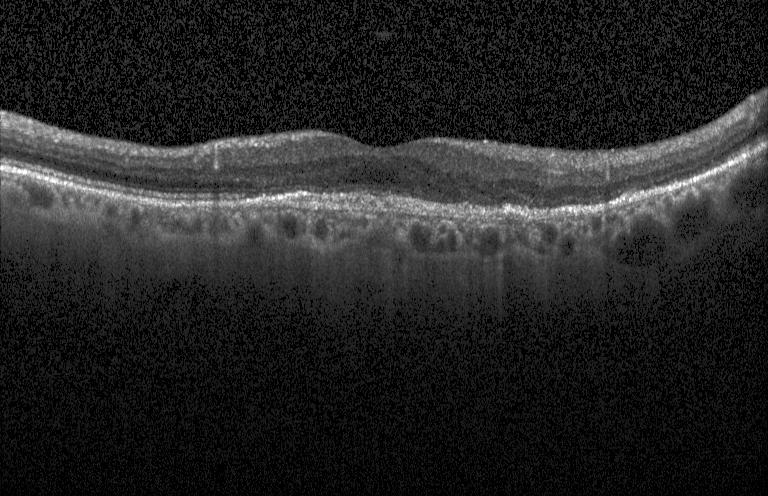

A choroidal neovascular membrane.